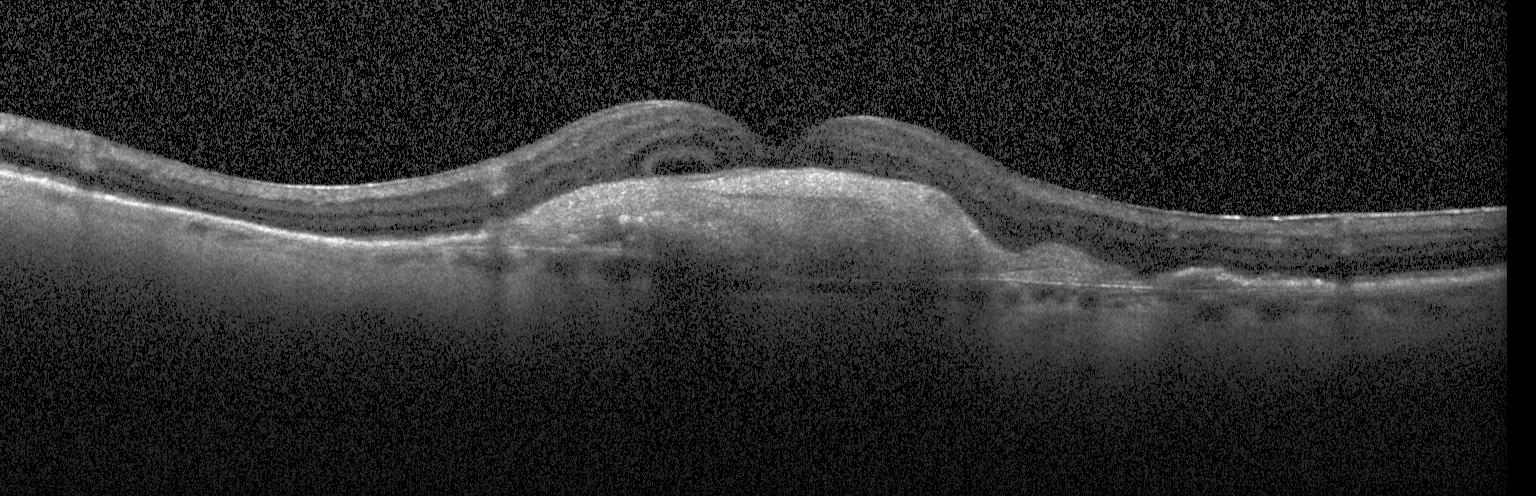 SD-OCT · retinal OCT B-scan · centered on the fovea · Heidelberg Spectralis OCT system
Finding: a choroidal neovascular membrane.